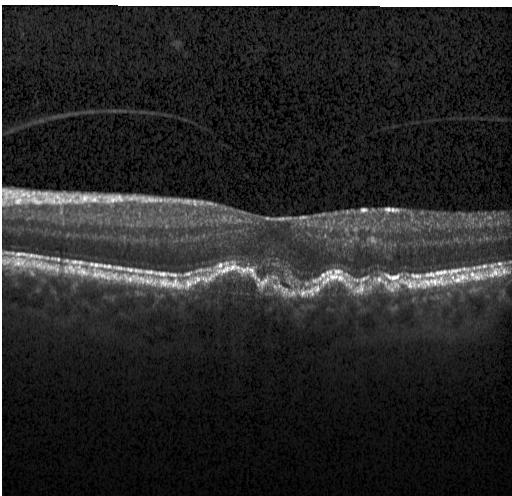 Retinal OCT cross-section.
Dx: multiple drusen.